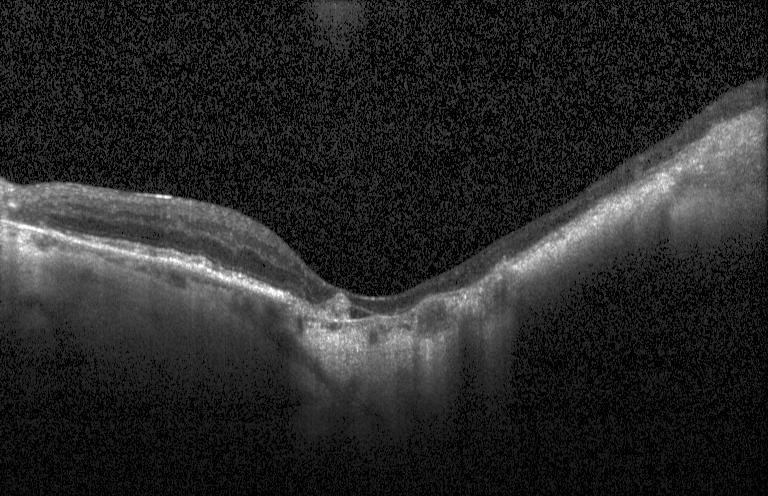
Spectral-domain OCT B-scan: choroidal neovascularization.